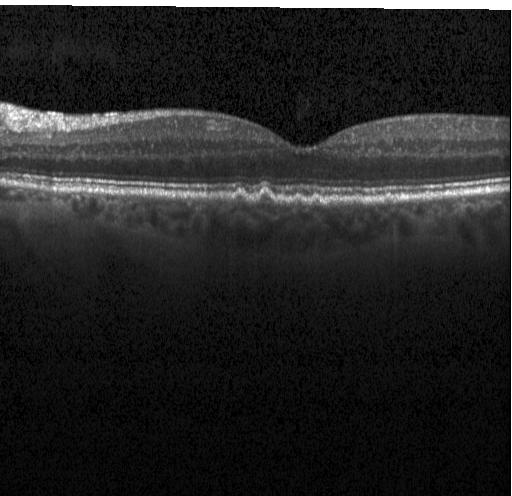 Multiple drusen.